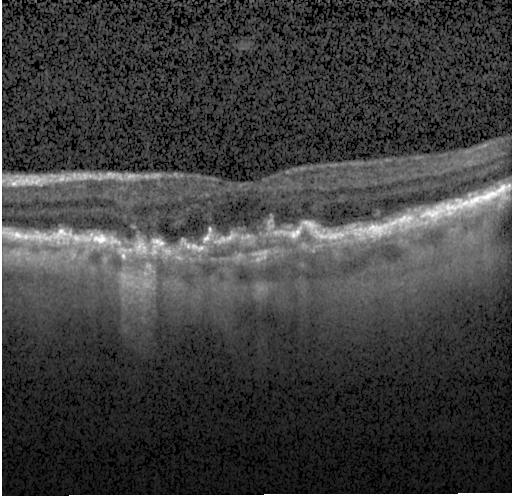
Retinal OCT cross-section.
Diagnosis: choroidal neovascularization (CNV).